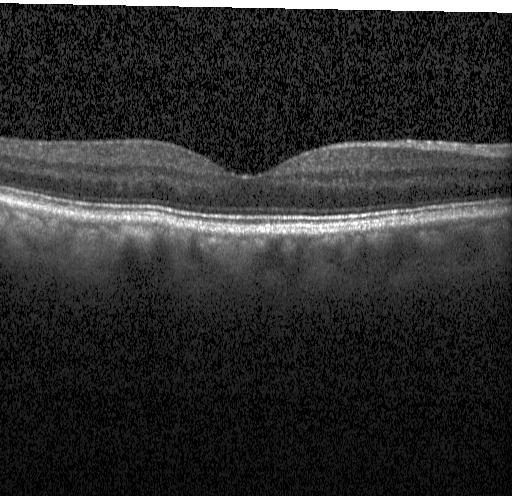
Spectral-domain OCT B-scan: neither CNV, DME, nor drusen.